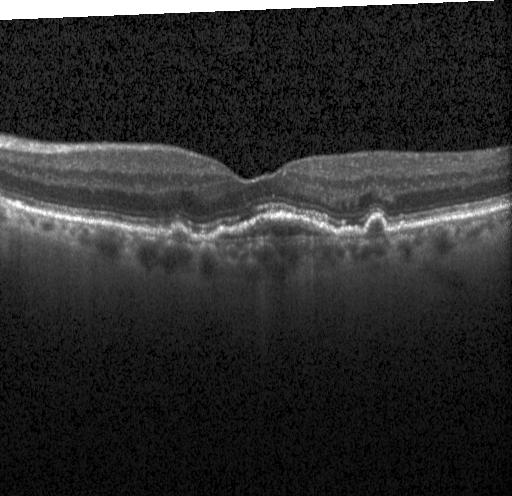 SD-OCT · acquired on a Heidelberg Spectralis · optical coherence tomography B-scan — Dx: a choroidal neovascular membrane.